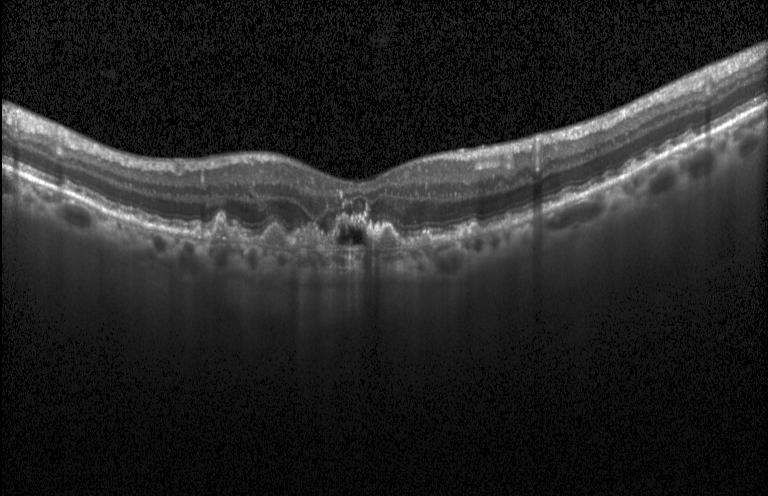

Finding: CNV.